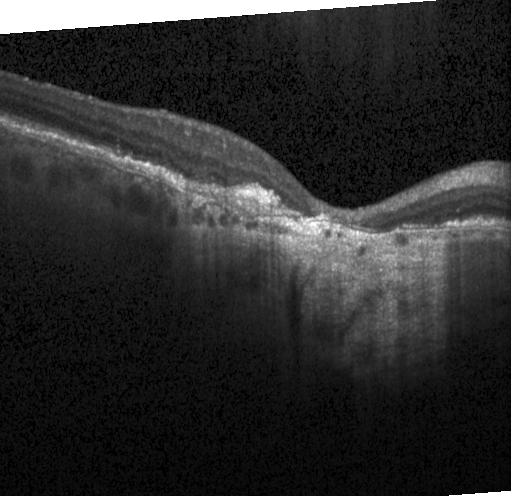

Diagnosis: a choroidal neovascular membrane.